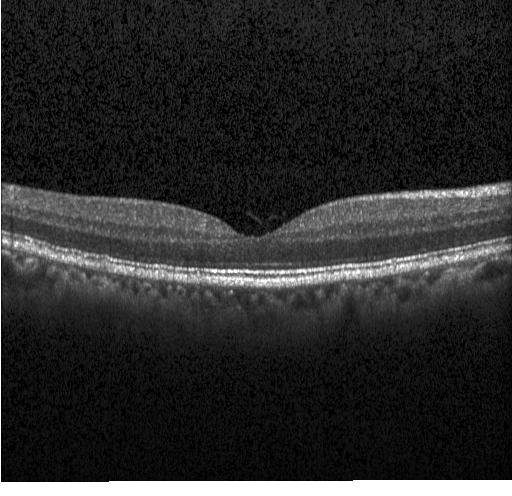
OCT B-scan · Heidelberg Spectralis — The scan shows no evidence of choroidal neovascularization, diabetic macular edema, or drusen.